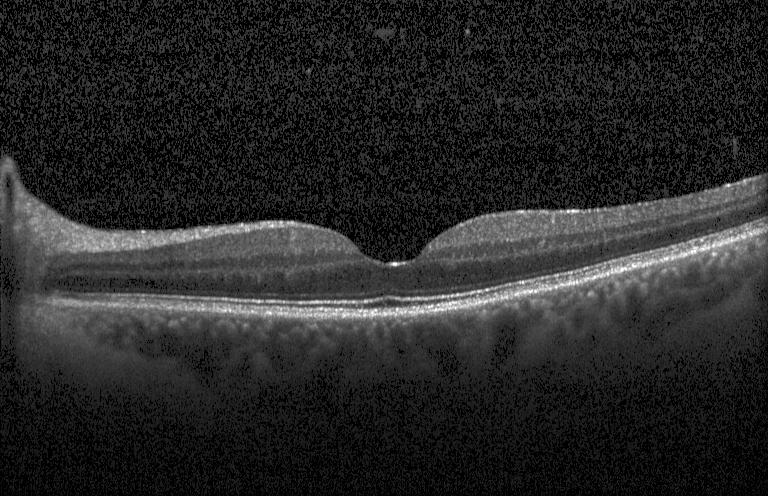

Spectral-domain optical coherence tomography; fovea-centered; retinal OCT B-scan; acquired on a Heidelberg Spectralis
The scan shows no choroidal neovascularization, no diabetic macular edema, and no drusen.